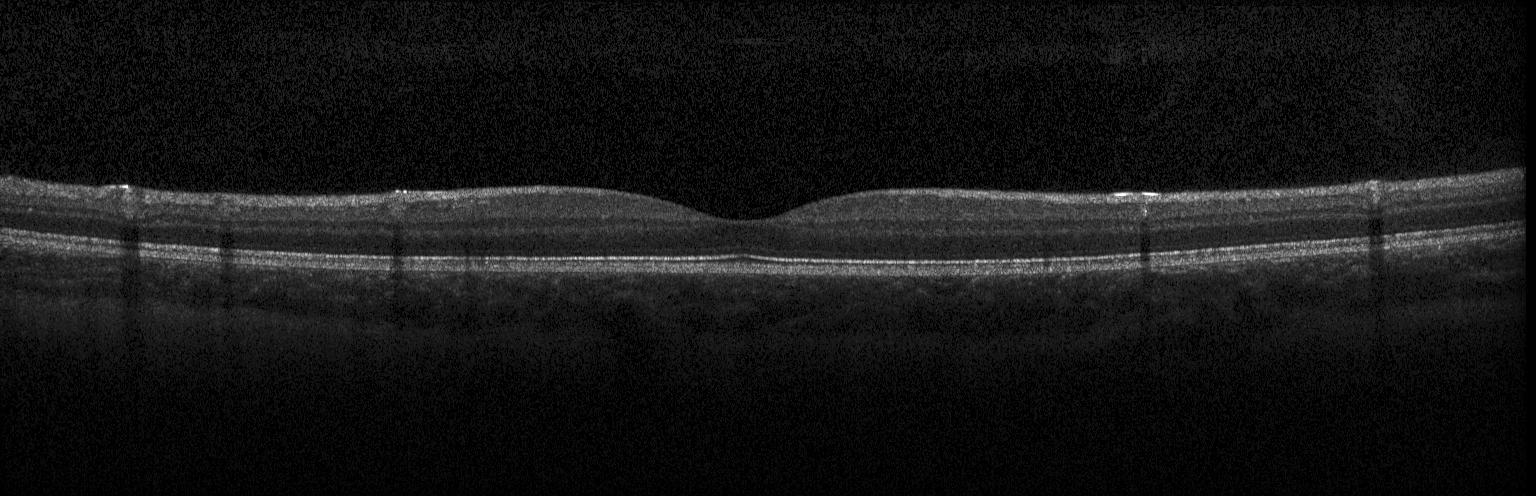
Neither choroidal neovascularization, diabetic macular edema, nor drusen.